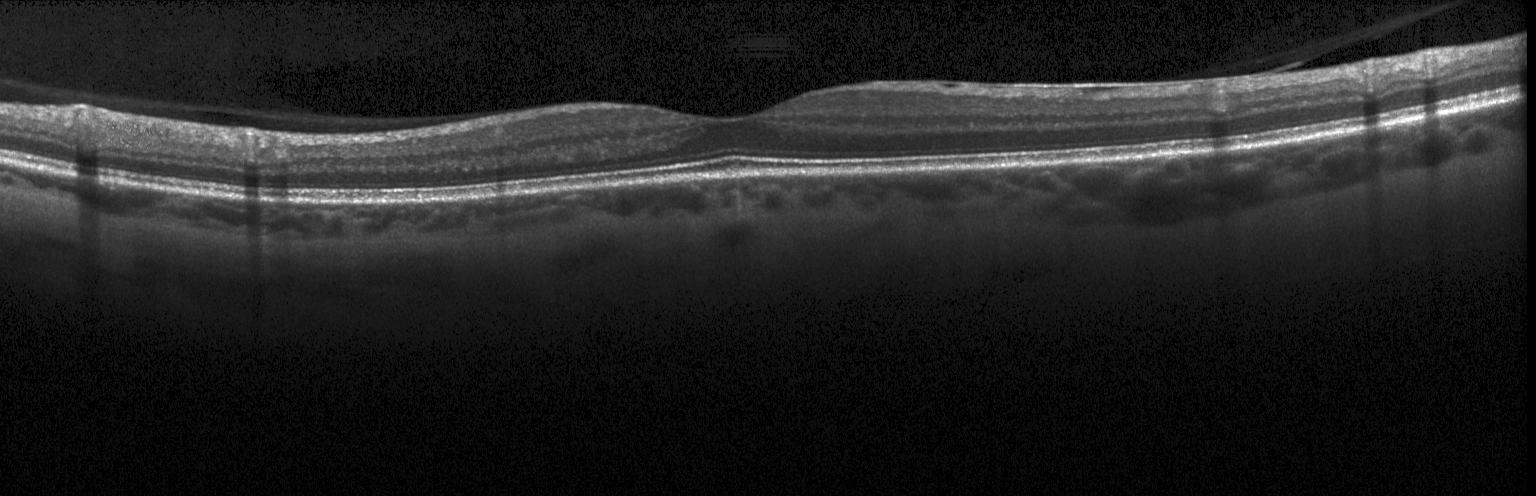
Optical coherence tomography scan · spectral-domain optical coherence tomography · Heidelberg Spectralis OCT system. Neither choroidal neovascularization, diabetic macular edema, nor drusen.